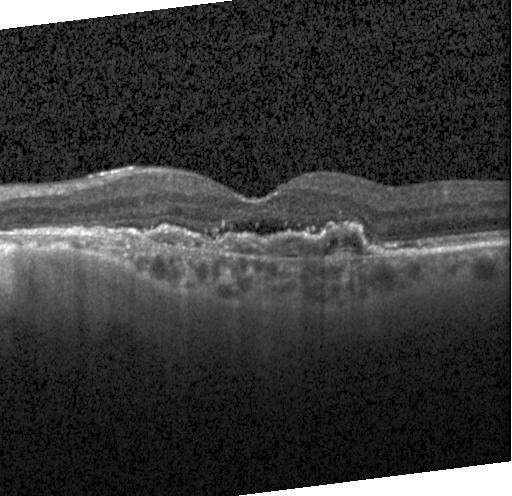
OCT B-scan · fovea-centered.
Macular OCT: choroidal neovascularization (CNV).